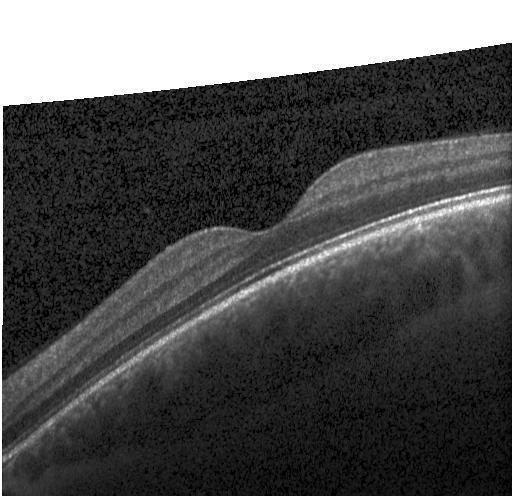

Spectral-domain OCT; fovea-centered; optical coherence tomography scan
The scan shows no evidence of choroidal neovascularization, diabetic macular edema, or drusen.